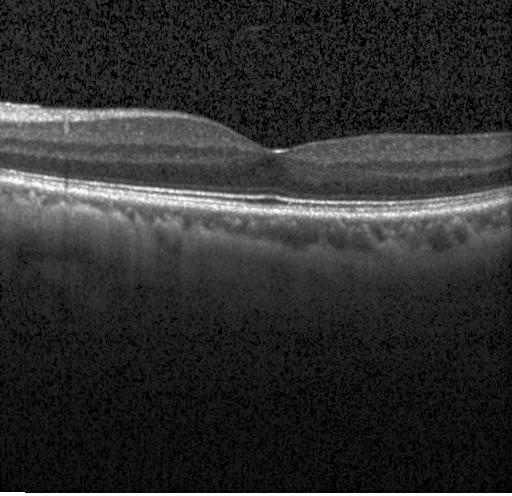
Impression: neither CNV, DME, nor drusen.